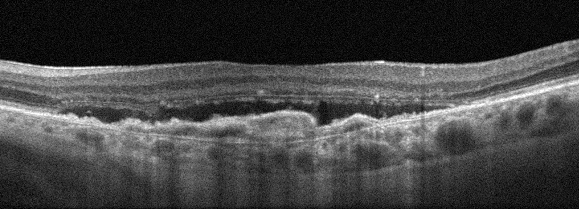 Optovue Avanti RTVue XR · left eye · OCT line scan
Dx: AMD.